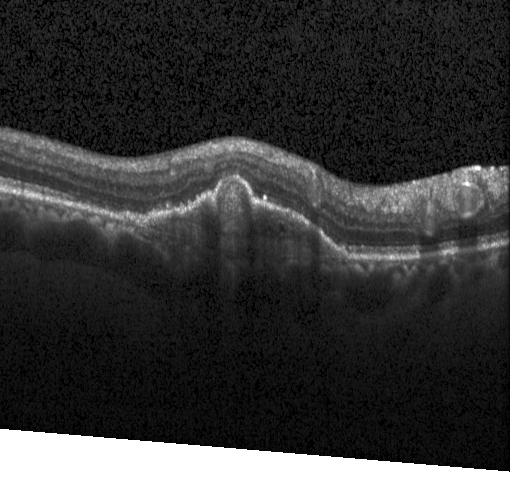

Impression: a choroidal neovascular membrane.